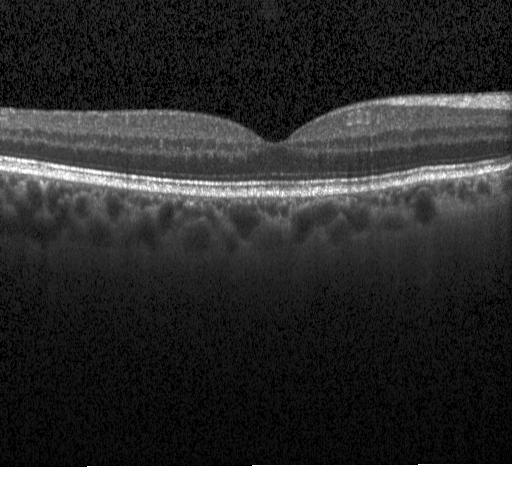 No choroidal neovascularization, diabetic macular edema, or drusen.